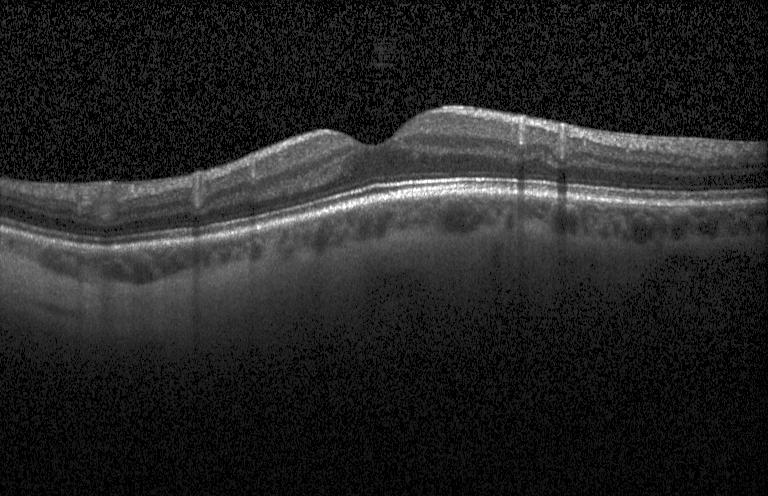

Retinal OCT B-scan · spectral-domain optical coherence tomography · fovea-centered.
Dx: no choroidal neovascularization, no diabetic macular edema, and no drusen.